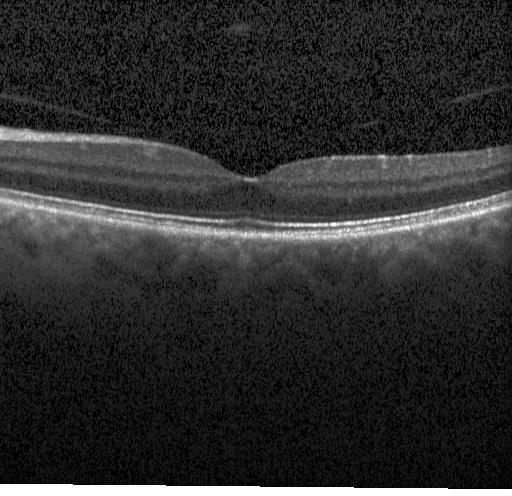 OCT finding: no choroidal neovascularization, diabetic macular edema, or drusen.